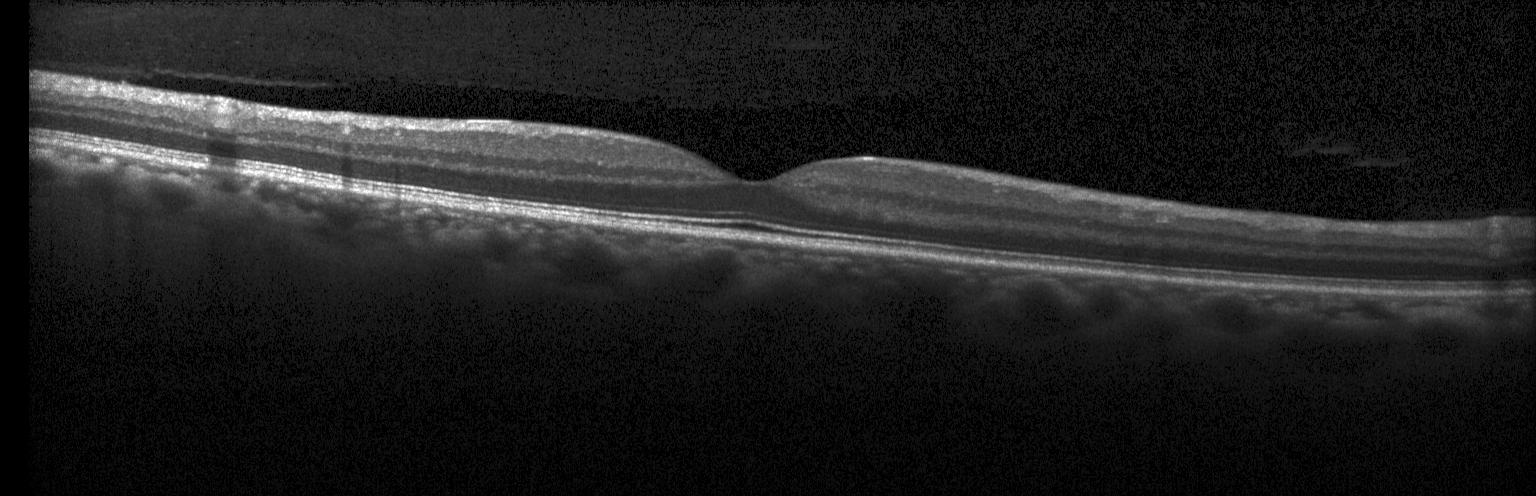

OCT line scan — Finding: no choroidal neovascularization, no diabetic macular edema, and no drusen.